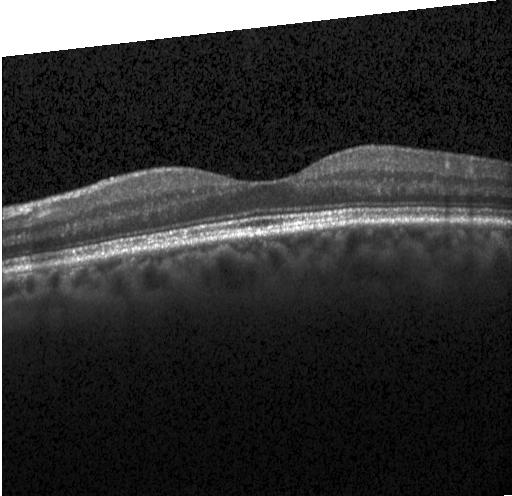

SD-OCT; OCT B-scan; Heidelberg Spectralis OCT system; centered on the fovea — Finding: no evidence of choroidal neovascularization, diabetic macular edema, or drusen.